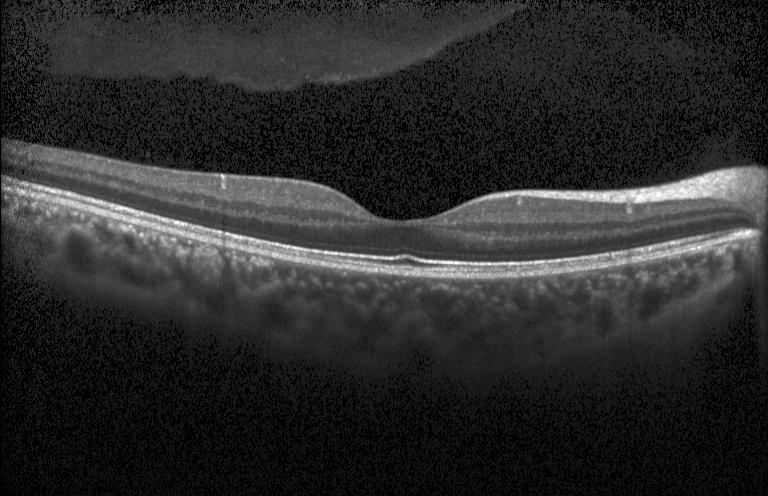 OCT line scan. No evidence of choroidal neovascularization, diabetic macular edema, or drusen.